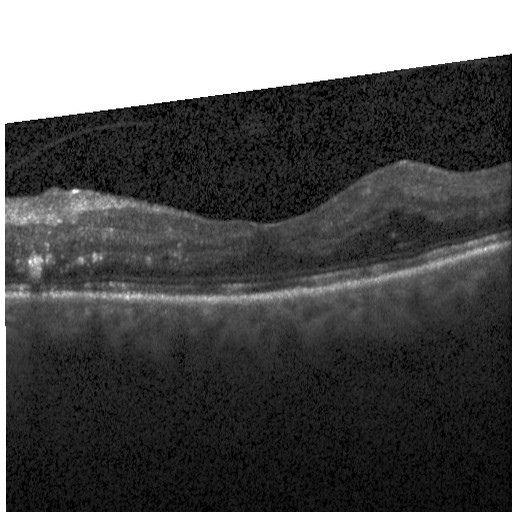

Optical coherence tomography B-scan. Spectral-domain optical coherence tomography. Acquired on a Heidelberg Spectralis.
This B-scan demonstrates DME.